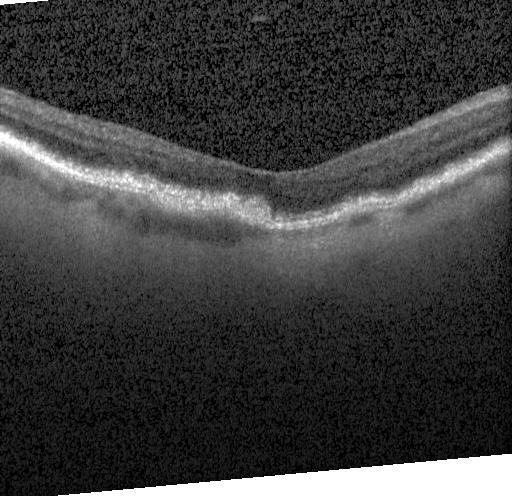 Heidelberg Spectralis OCT system, SD-OCT, centered on the fovea, retinal OCT B-scan
Impression: a choroidal neovascular membrane.